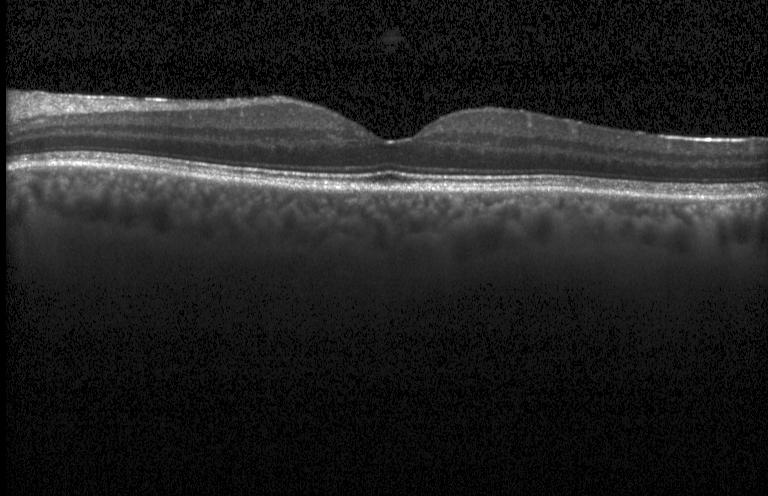
Spectral-domain OCT B-scan: no choroidal neovascularization, no diabetic macular edema, and no drusen.